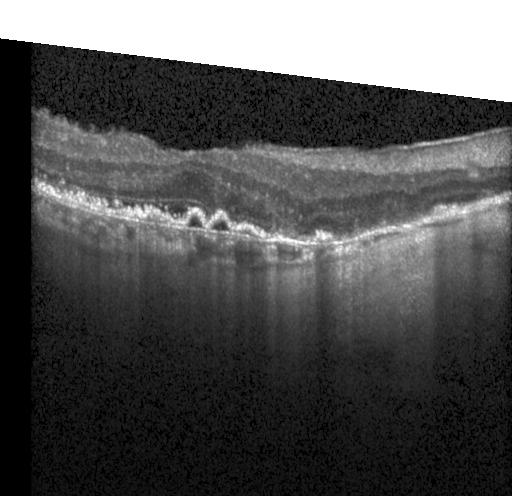
OCT B-scan showing CNV.